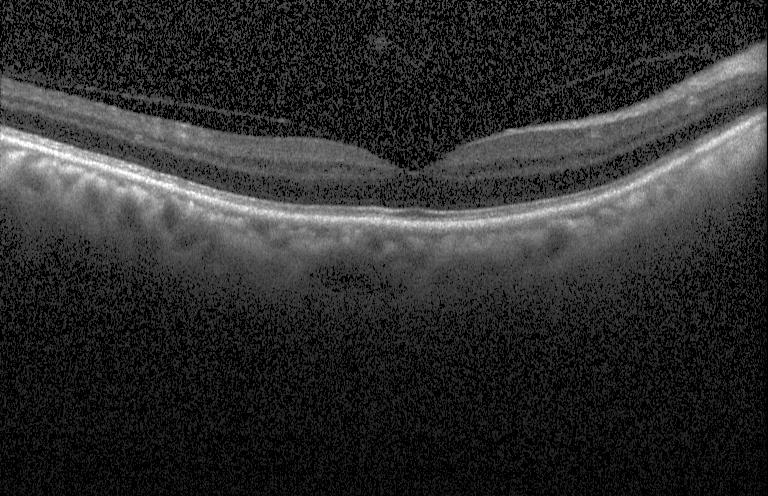 OCT scan showing no evidence of choroidal neovascularization, diabetic macular edema, or drusen.